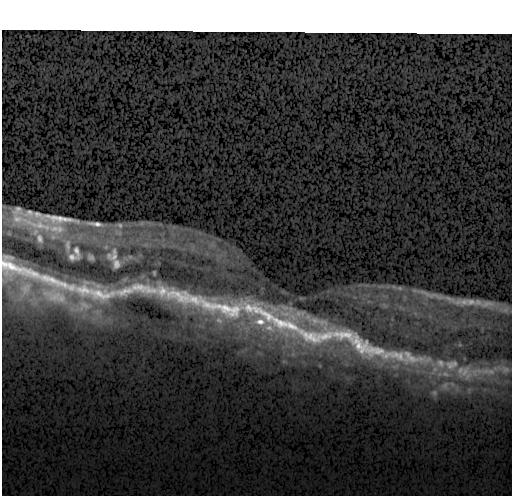

This B-scan demonstrates a choroidal neovascular membrane.